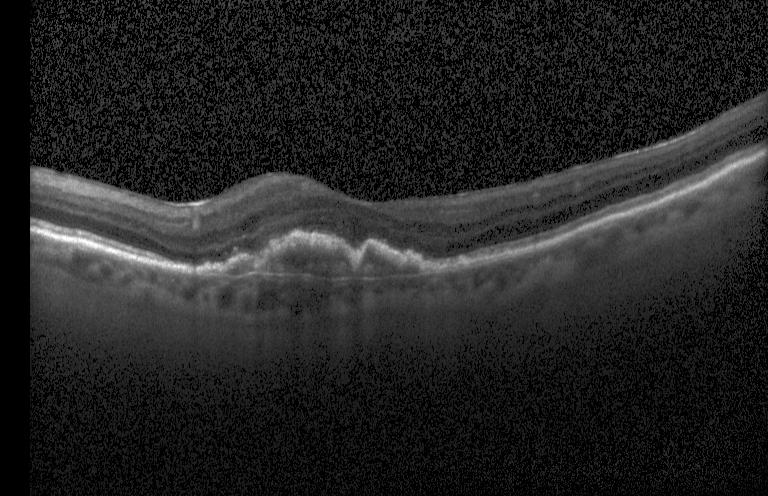 This B-scan demonstrates a choroidal neovascular membrane.